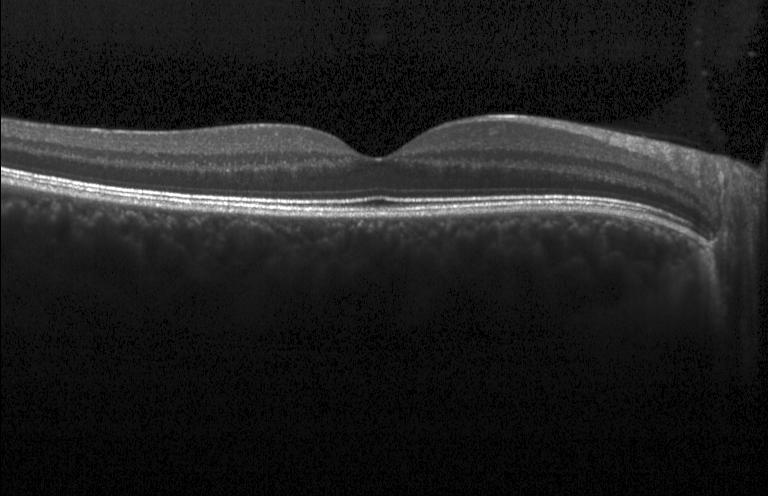

Fovea-centered · Heidelberg Spectralis · optical coherence tomography scan — Dx: neither CNV, DME, nor drusen.